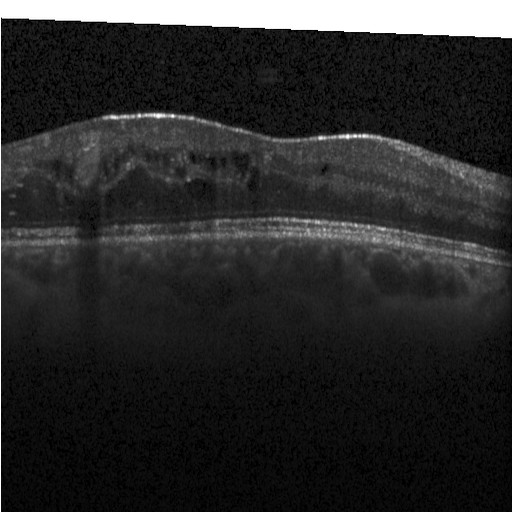

Retinal OCT B-scan — Finding: diabetic macular edema.